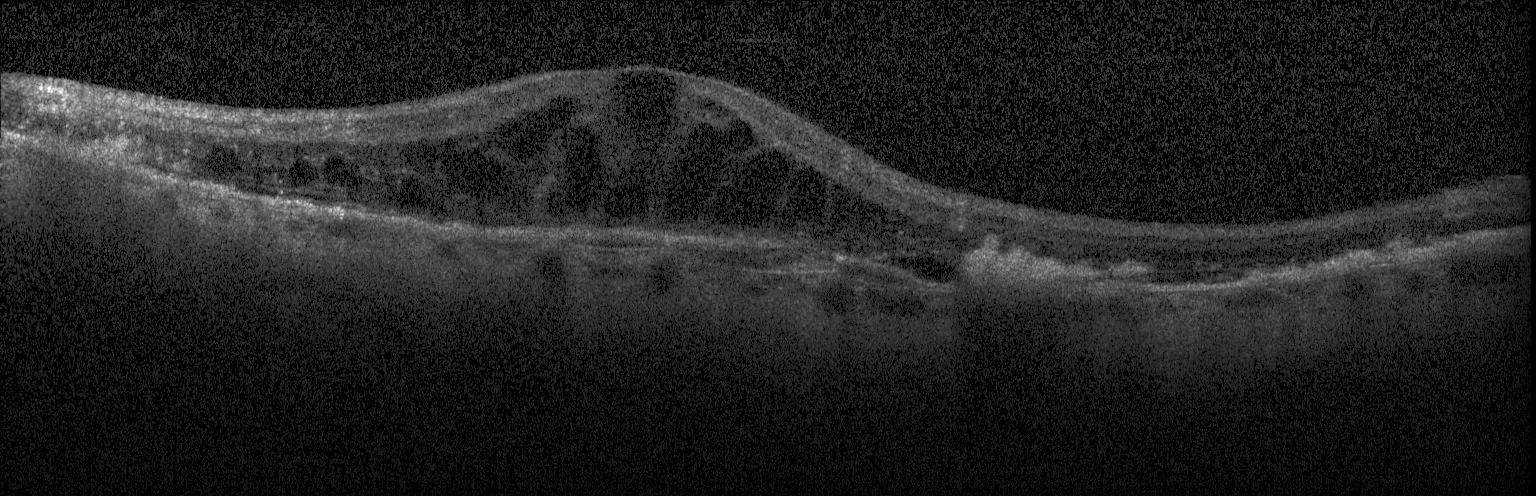
OCT line scan. Impression: choroidal neovascularization (CNV).